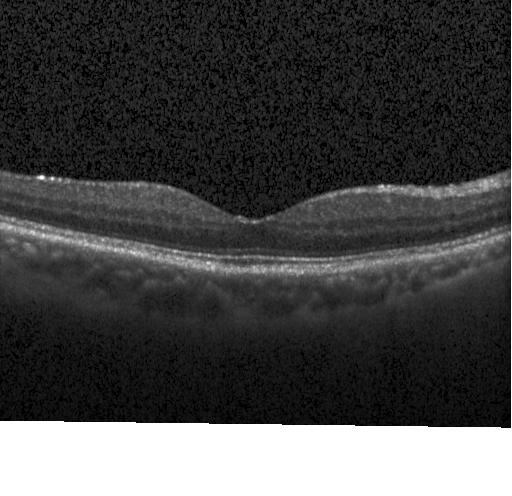

Retinal OCT cross-section; Heidelberg Spectralis OCT system; fovea-centered; SD-OCT
Finding: neither CNV, DME, nor drusen.